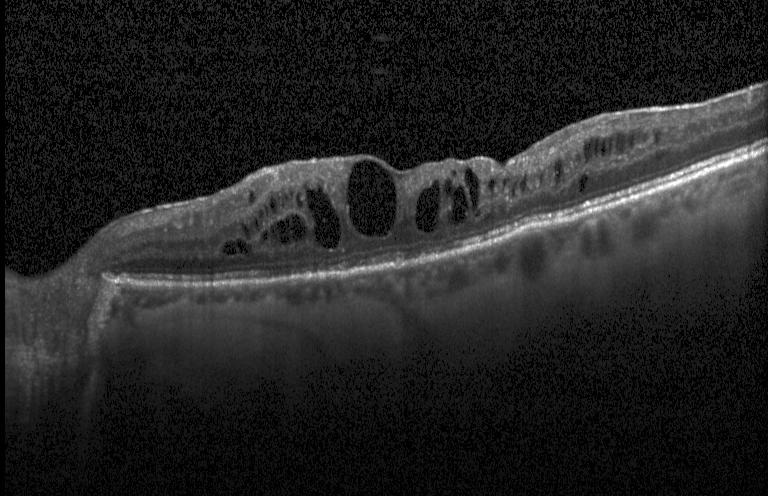

This B-scan demonstrates DME.